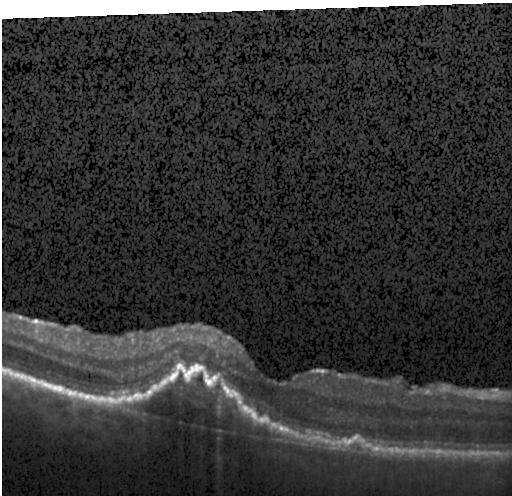

Macular OCT: a choroidal neovascular membrane.